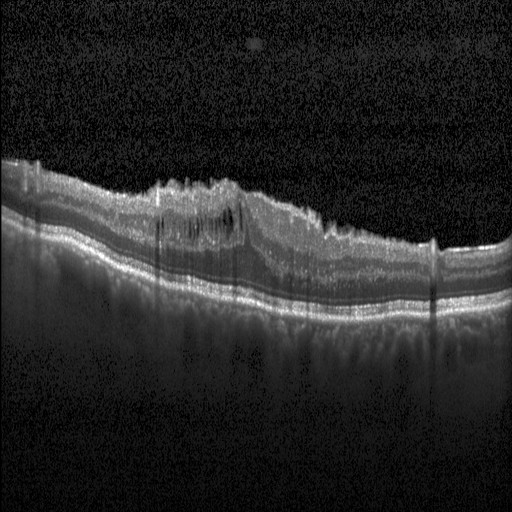

Diagnosis: DME.